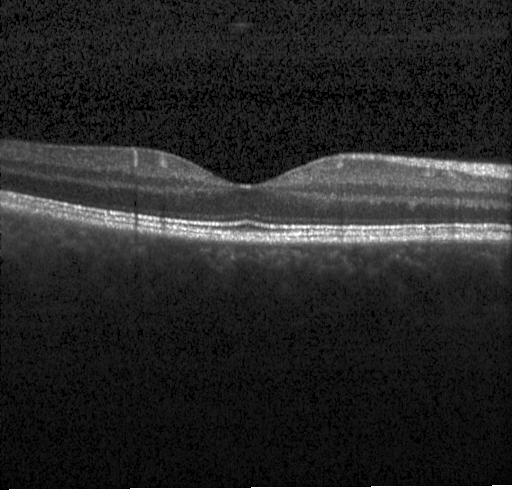 Diagnosis: neither choroidal neovascularization, diabetic macular edema, nor drusen.